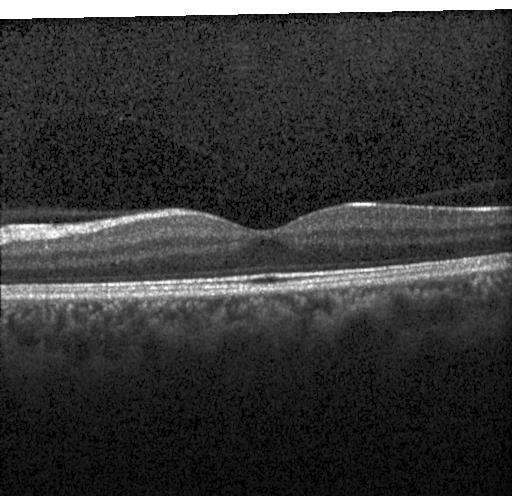
Retinal OCT cross-section showing no CNV, no DME, and no drusen.